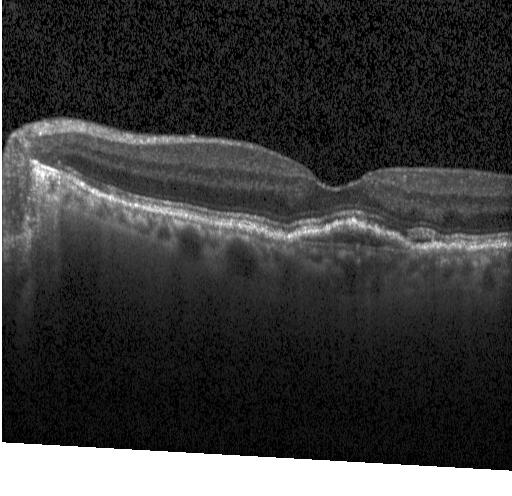

Fovea-centered · SD-OCT · retinal OCT B-scan. Finding: a choroidal neovascular membrane.